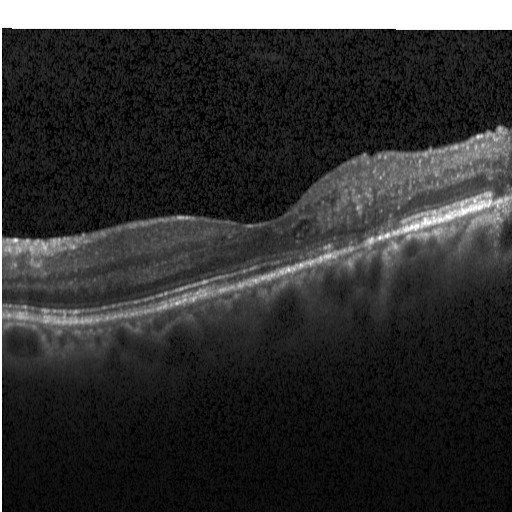

OCT line scan. Finding: DME.